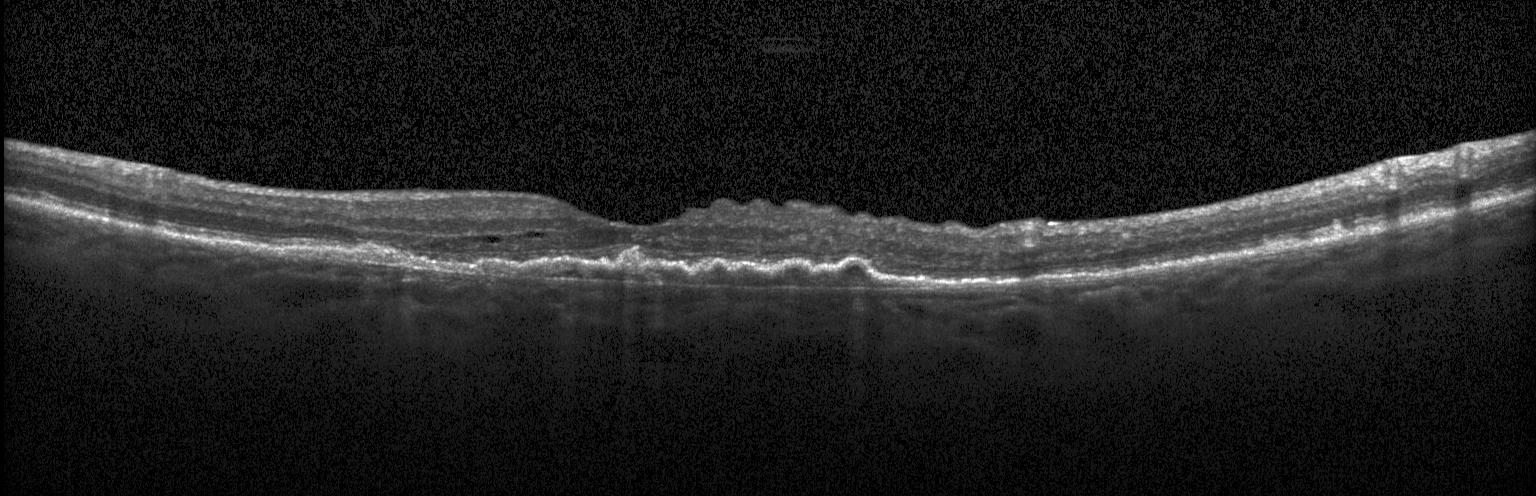

Through the macula; optical coherence tomography B-scan — Diagnosis: a choroidal neovascular membrane.